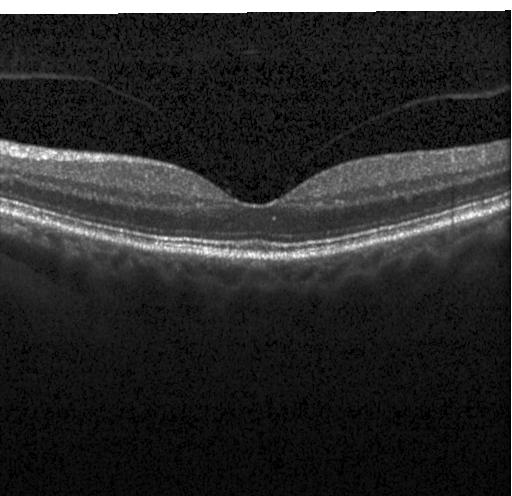
Finding: no choroidal neovascularization, no diabetic macular edema, and no drusen.